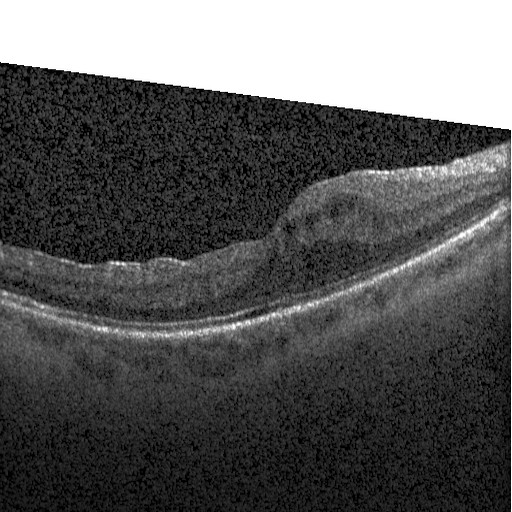
Diagnosis: diabetic macular edema.